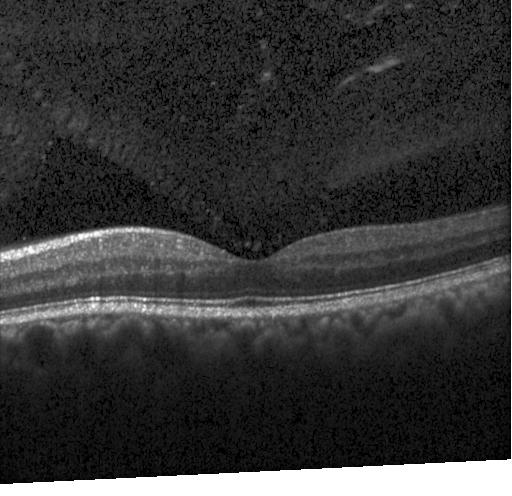

SD-OCT; retinal OCT B-scan.
Dx: no evidence of choroidal neovascularization, diabetic macular edema, or drusen.